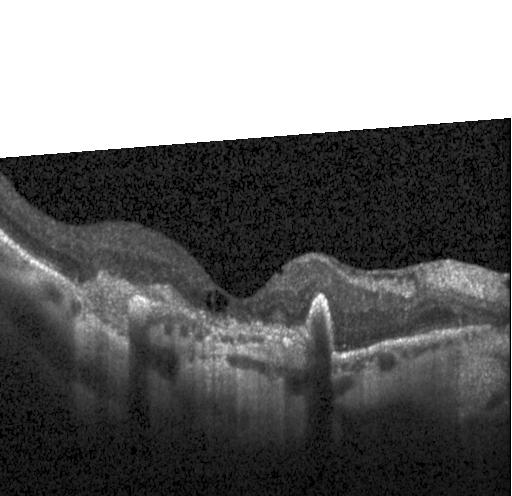
Macular OCT: a choroidal neovascular membrane.